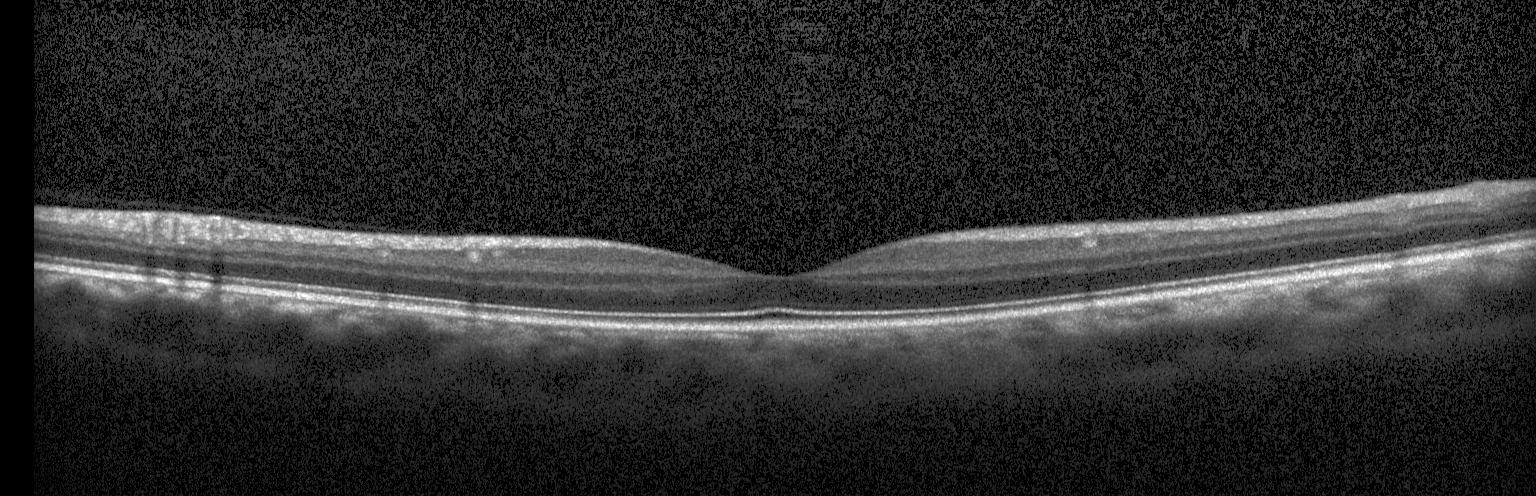 Spectral-domain OCT; centered on the fovea; optical coherence tomography B-scan; Heidelberg Spectralis.
Impression: no CNV, no DME, and no drusen.